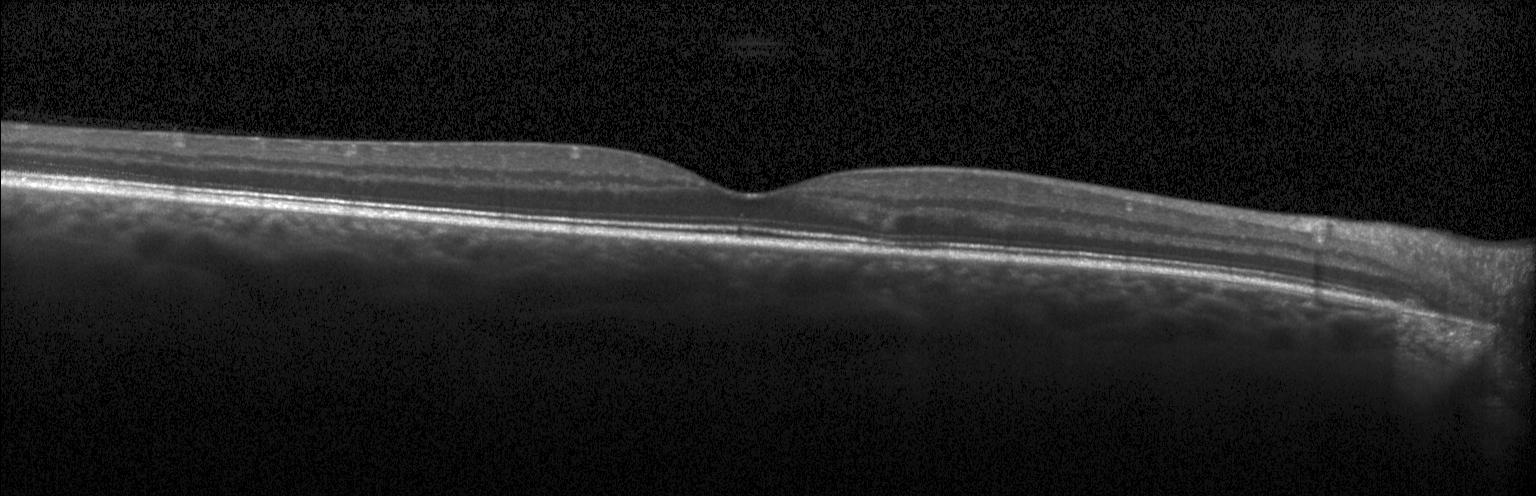
Finding: no choroidal neovascularization, no diabetic macular edema, and no drusen.